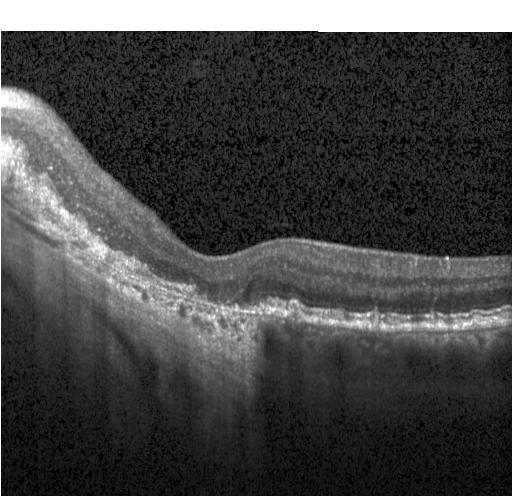

Diagnosis: a choroidal neovascular membrane.